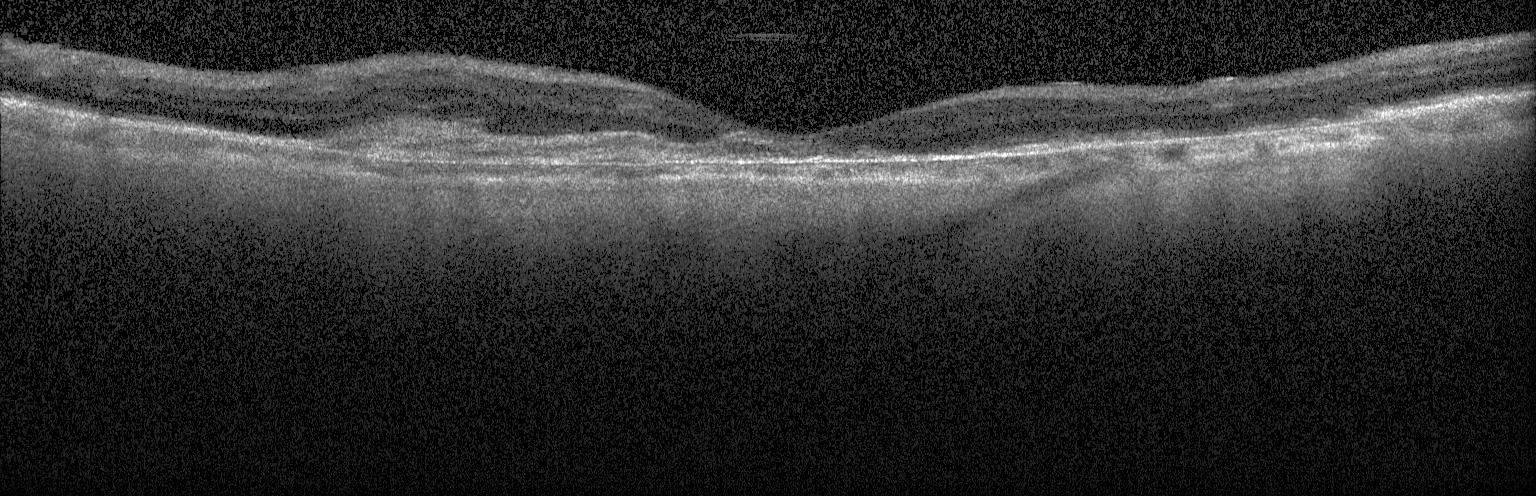
Acquired on a Heidelberg Spectralis. OCT B-scan
Impression: CNV.